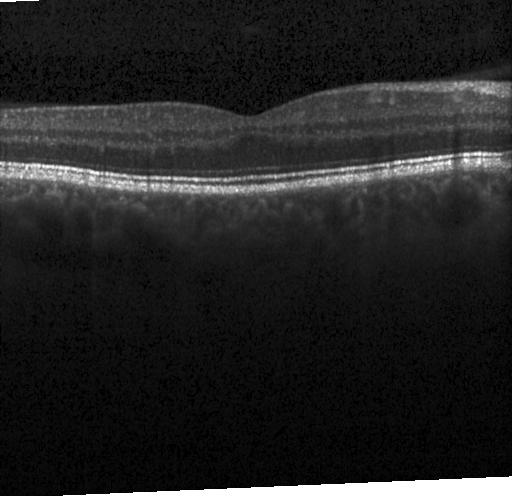
The scan shows no evidence of choroidal neovascularization, diabetic macular edema, or drusen.